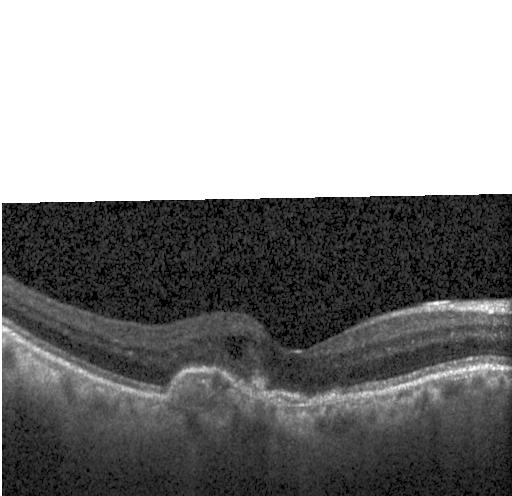

Retinal OCT B-scan. Spectral-domain optical coherence tomography. Heidelberg Spectralis. Centered on the fovea — Diagnosis: choroidal neovascularization.